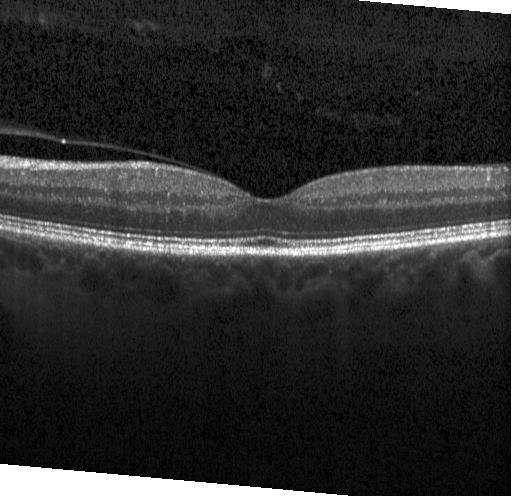 Macular OCT: neither choroidal neovascularization, diabetic macular edema, nor drusen.